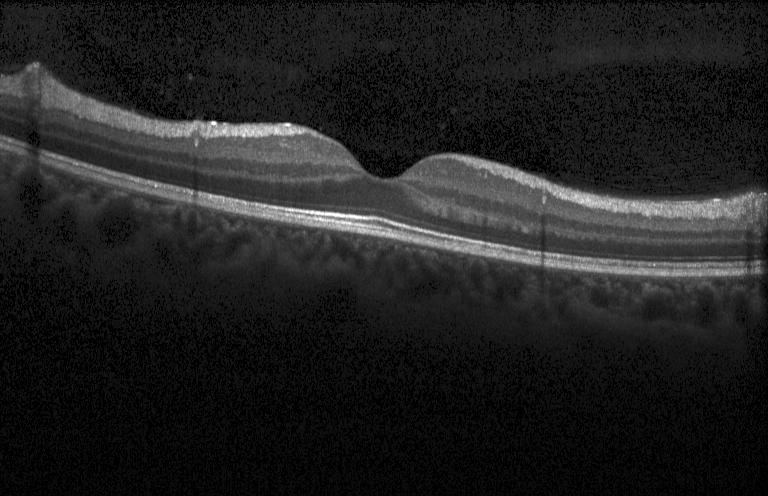
Heidelberg Spectralis, centered on the fovea, OCT line scan. Impression: no CNV, DME, or drusen.